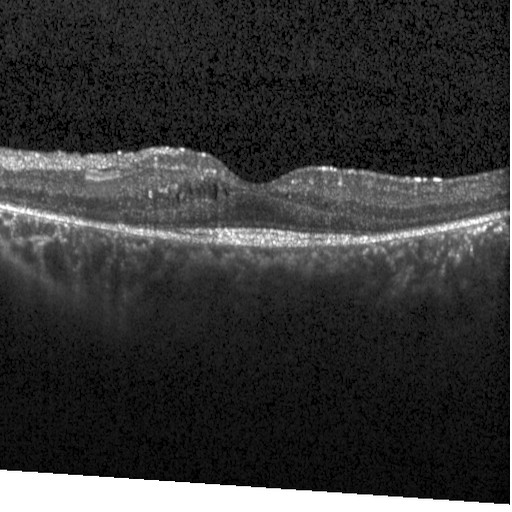
OCT line scan, SD-OCT, acquired on a Heidelberg Spectralis.
Dx: diabetic macular edema (DME).